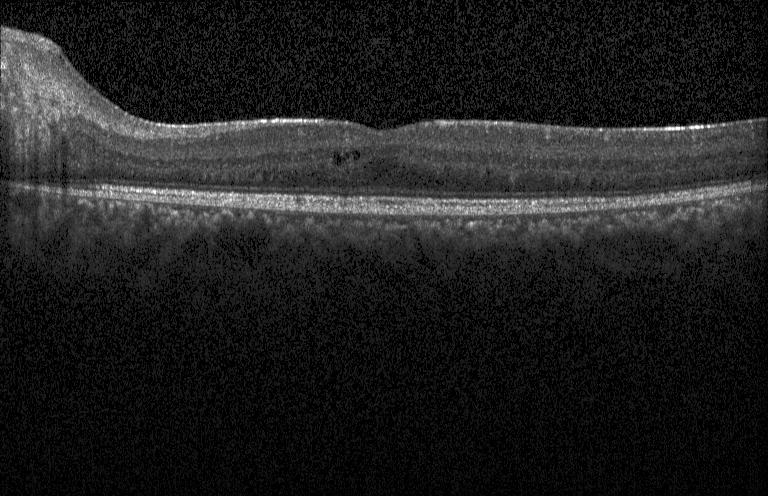
OCT B-scan, acquired on a Heidelberg Spectralis, through the macula, spectral-domain OCT — Finding: diabetic macular edema (DME).